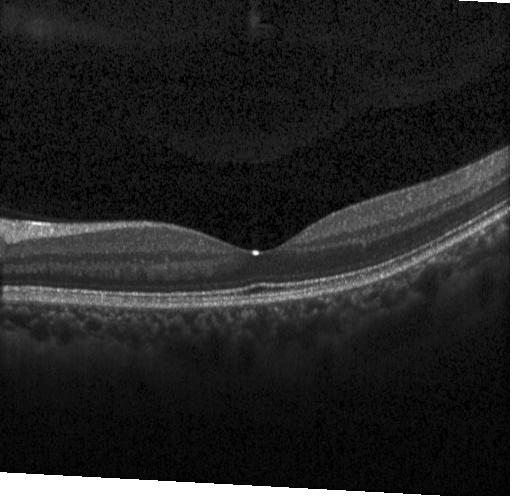
Retinal OCT B-scan; centered on the fovea; acquired on a Heidelberg Spectralis. Macular OCT: no evidence of CNV, DME, or drusen.